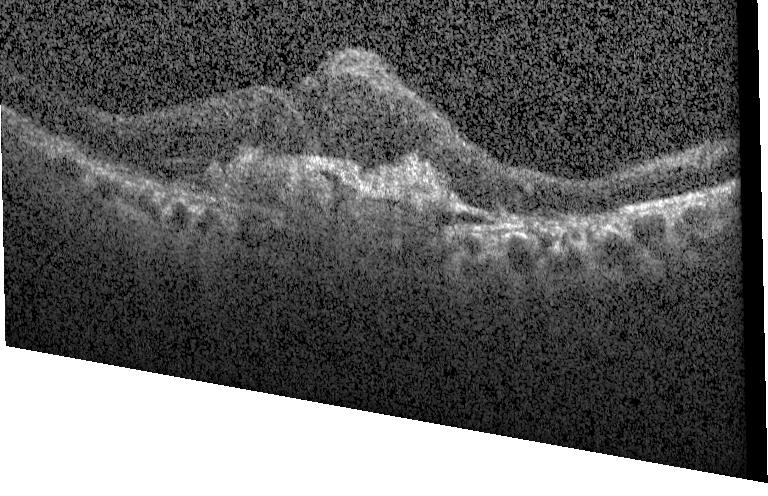 Centered on the fovea, optical coherence tomography scan — CNV.